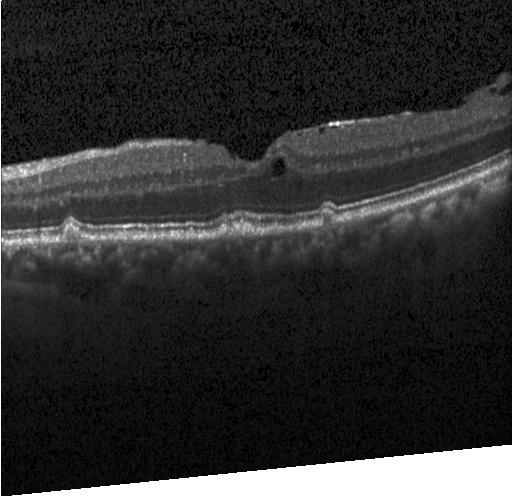
OCT scan showing drusen.